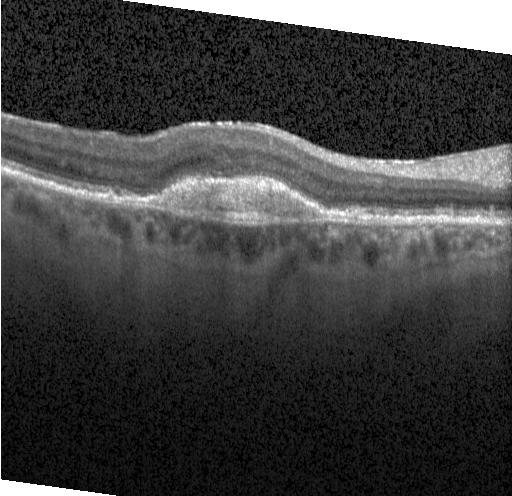
OCT B-scan
Dx: a choroidal neovascular membrane.